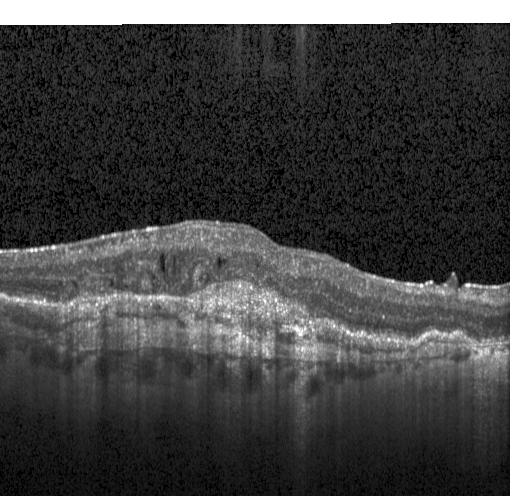 Assessment: a choroidal neovascular membrane.